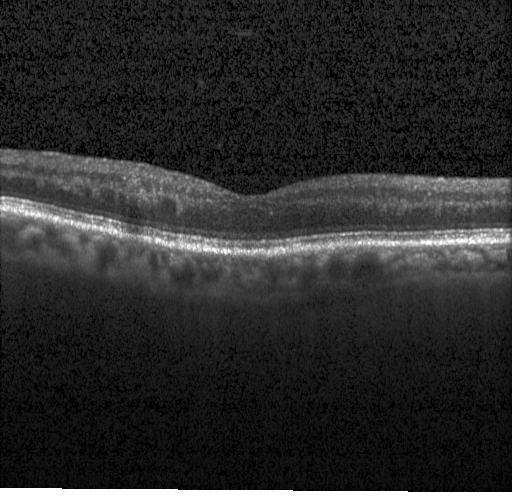

OCT B-scan. Heidelberg Spectralis. Horizontal scan through the fovea. Spectral-domain optical coherence tomography.
Diagnosis: no evidence of choroidal neovascularization, diabetic macular edema, or drusen.